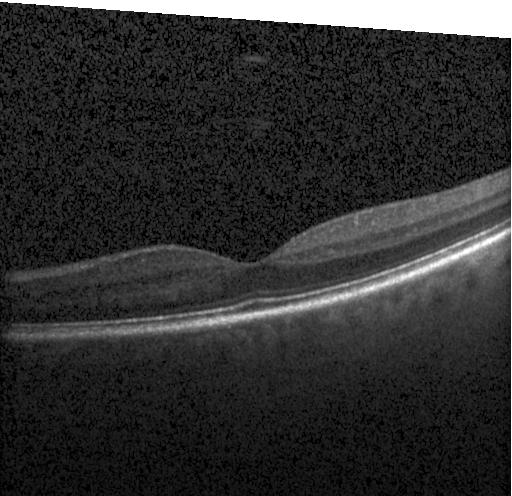

Macular OCT: no evidence of choroidal neovascularization, diabetic macular edema, or drusen.